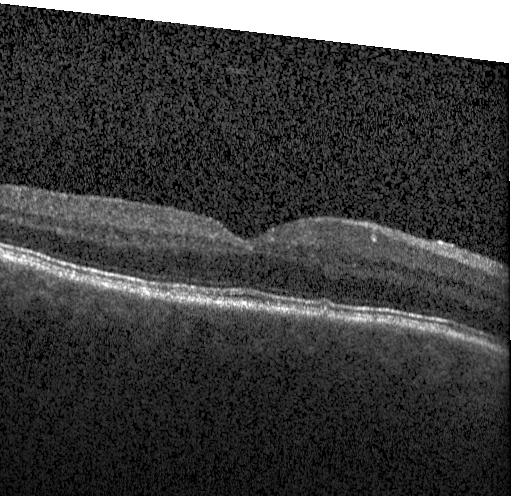 Retinal OCT cross-section — Macular OCT: neither CNV, DME, nor drusen.